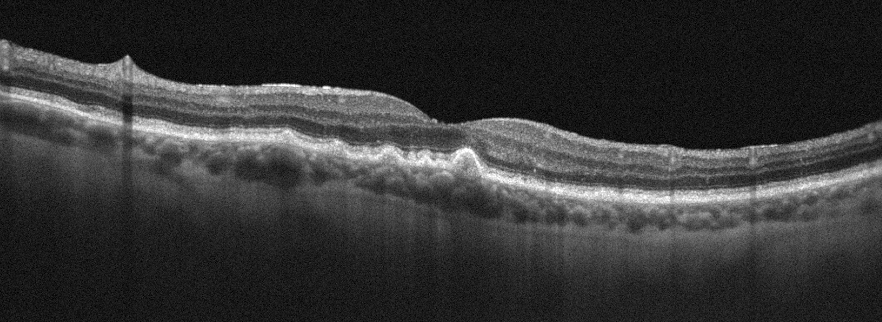

Macular OCT: age-related macular degeneration (AMD).